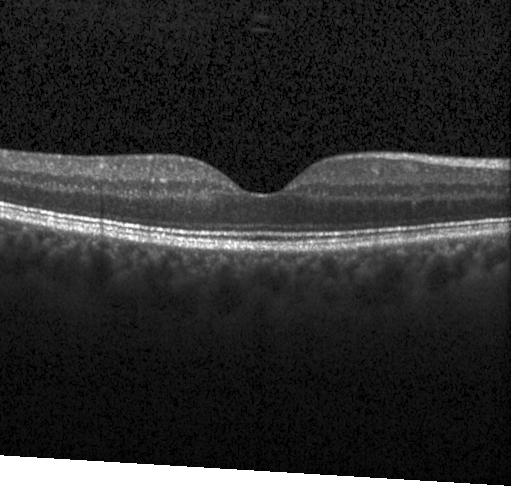
OCT B-scan showing neither CNV, DME, nor drusen.